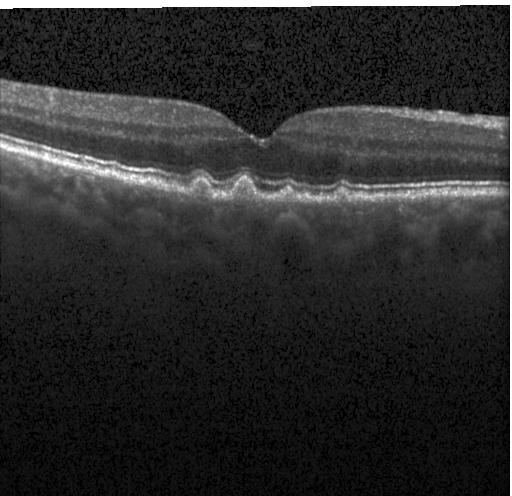
Assessment: drusen.